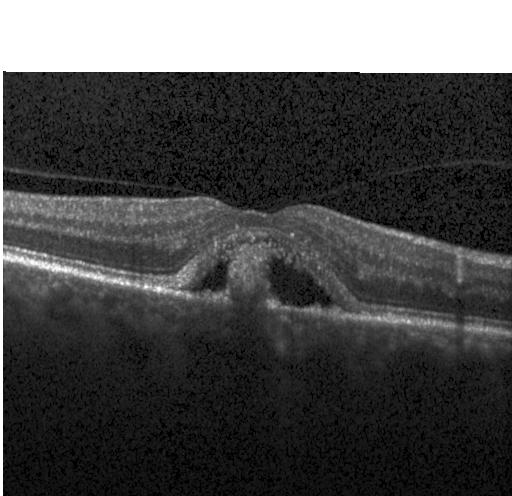 Retinal OCT cross-section — Diagnosis: a choroidal neovascular membrane.